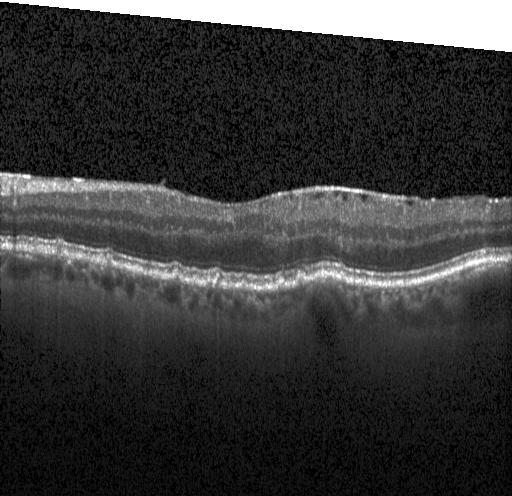

Diagnosis: sub-RPE drusenoid deposits.